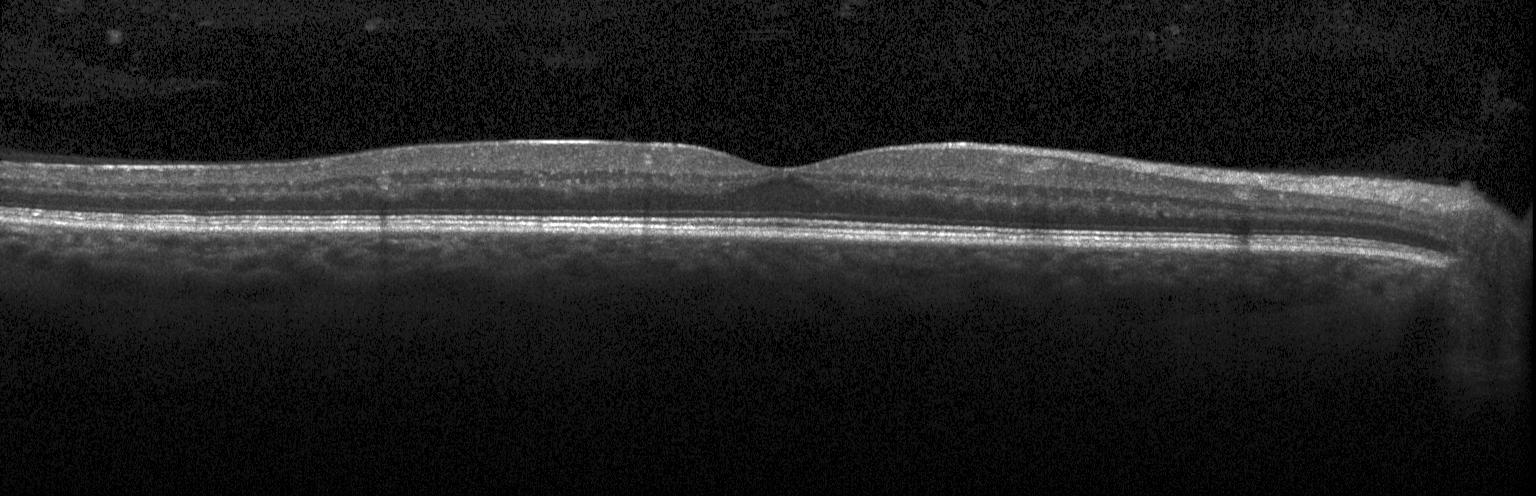
Spectral-domain optical coherence tomography · OCT B-scan
Finding: neither choroidal neovascularization, diabetic macular edema, nor drusen.